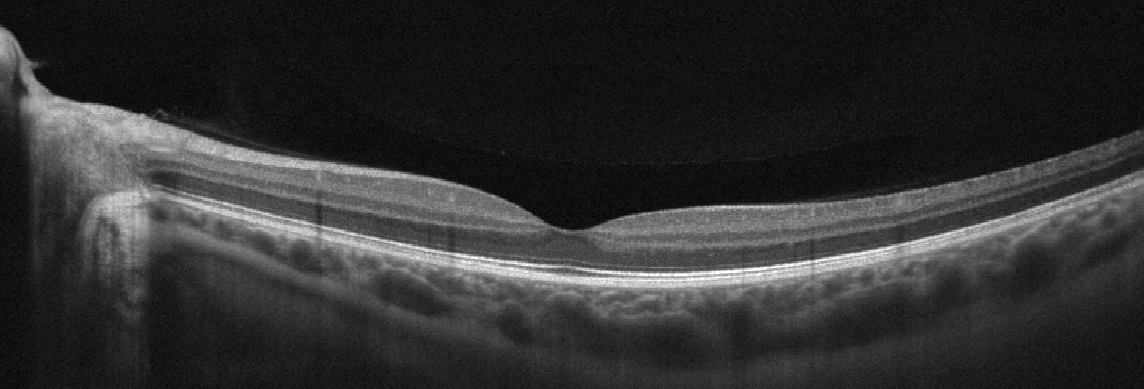
OCT line scan
Dx: absence of AMD, DME, ERM, RAO, RVO, and vitreomacular interface disease.